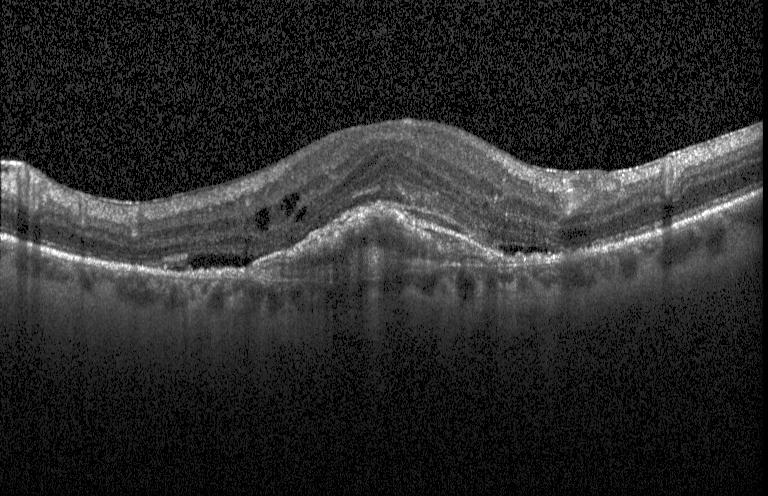
Assessment: CNV.